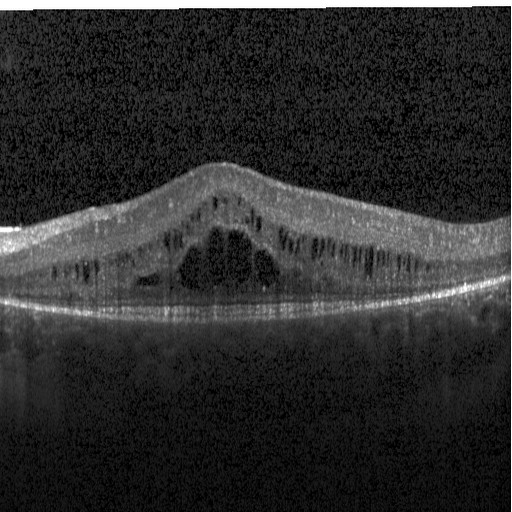 Optical coherence tomography scan · macular scan · instrument: Heidelberg Spectralis. The scan shows diabetic macular edema.